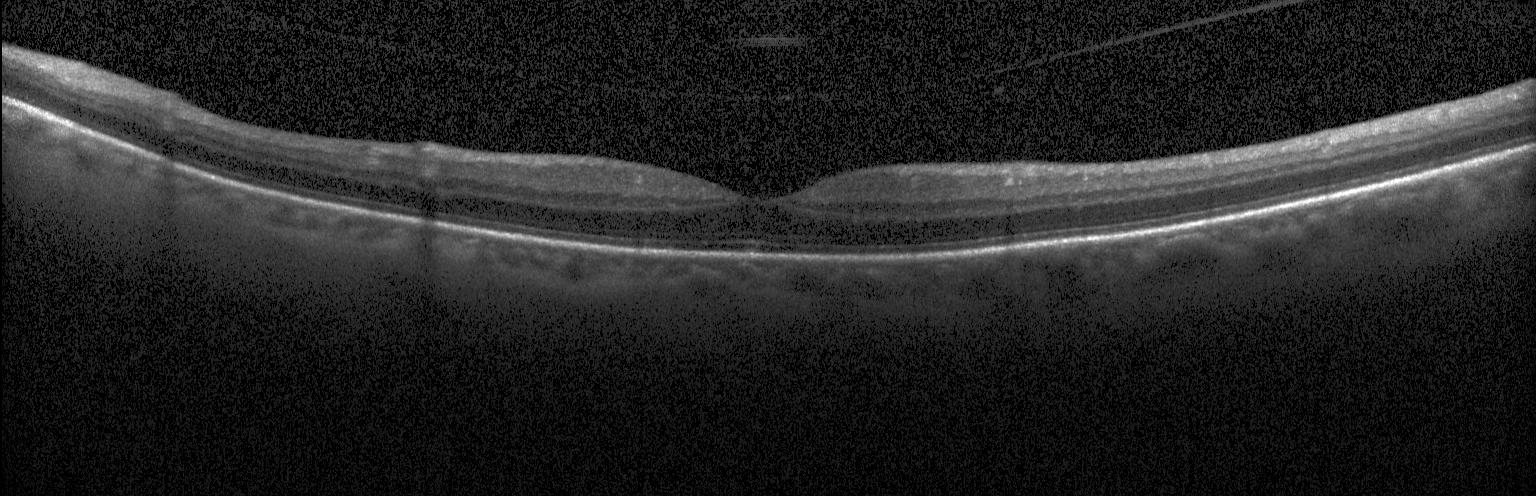
Retinal OCT B-scan; instrument: Heidelberg Spectralis; spectral-domain OCT. Finding: no CNV, DME, or drusen.